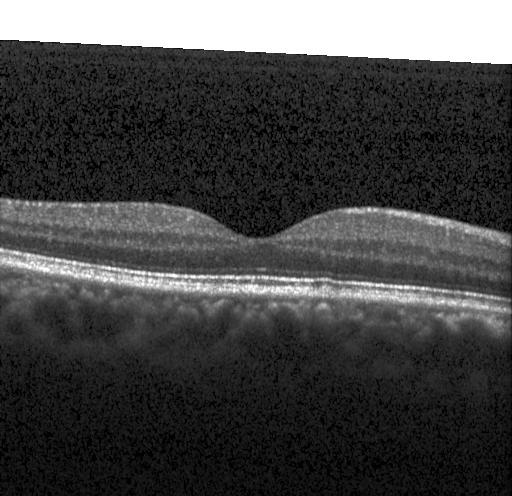 Retinal OCT B-scan · Heidelberg Spectralis · SD-OCT — Dx: no choroidal neovascularization, no diabetic macular edema, and no drusen.